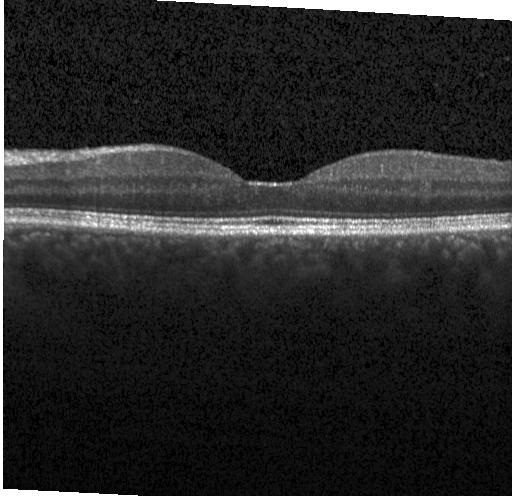
SD-OCT · optical coherence tomography scan — OCT finding: no CNV, no DME, and no drusen.